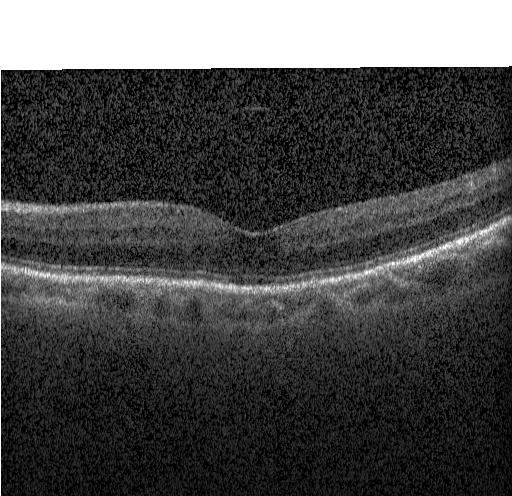
OCT B-scan showing no choroidal neovascularization, diabetic macular edema, or drusen.